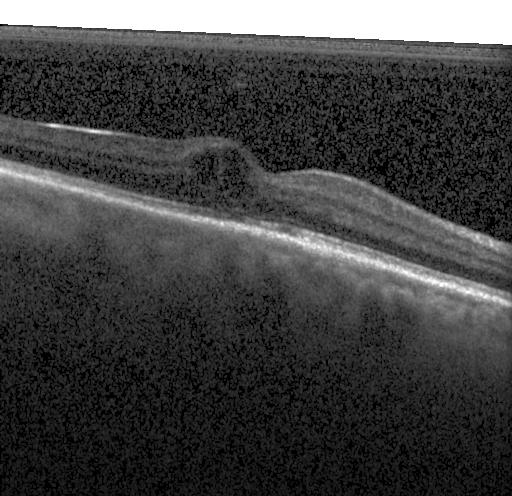
Assessment: DME.